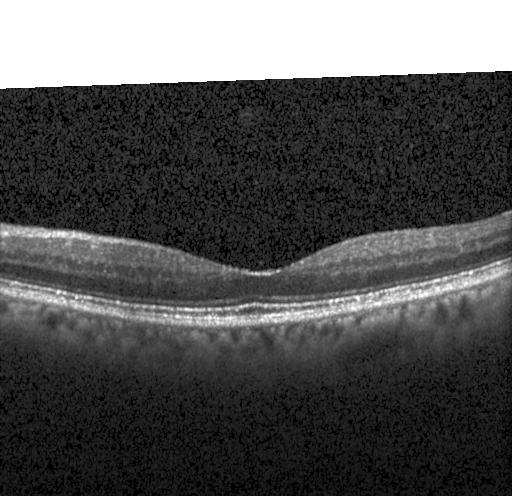

Spectral-domain optical coherence tomography, OCT line scan.
Diagnosis: neither CNV, DME, nor drusen.